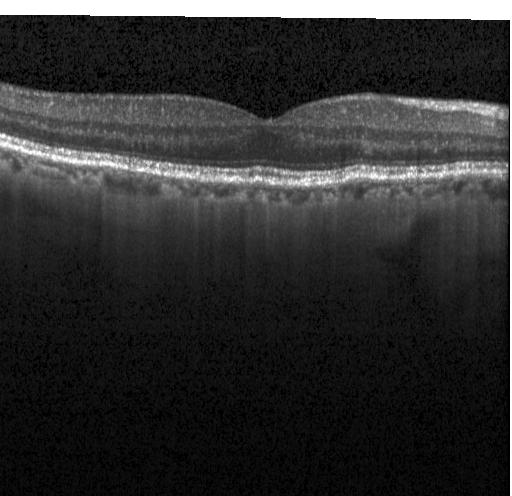
Macular scan. Spectral-domain OCT. Optical coherence tomography B-scan. Impression: sub-RPE drusenoid deposits.